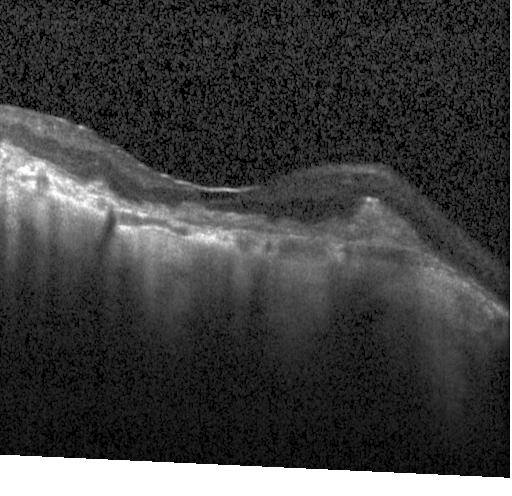

Impression: a choroidal neovascular membrane.